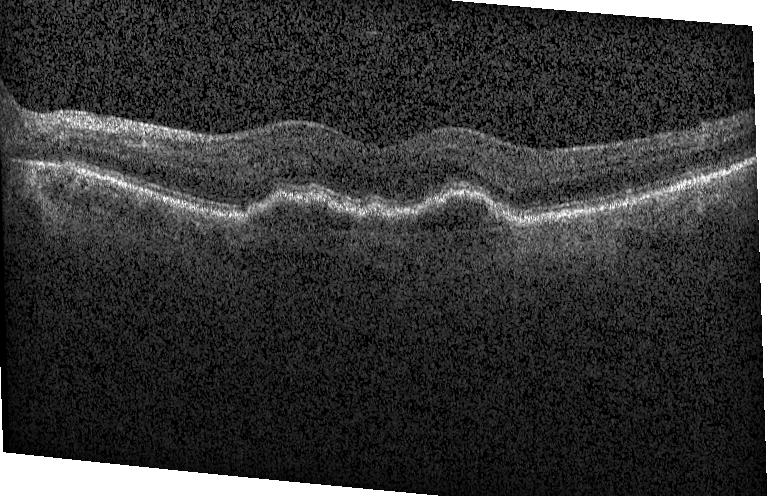
SD-OCT. Retinal OCT B-scan. Heidelberg Spectralis OCT system — Finding: a choroidal neovascular membrane.